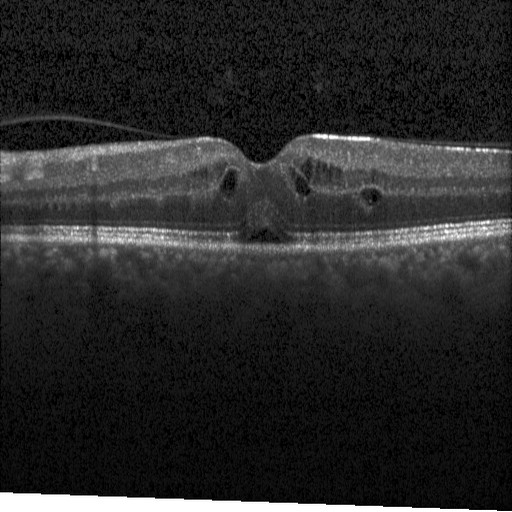
Diagnosis: DME.